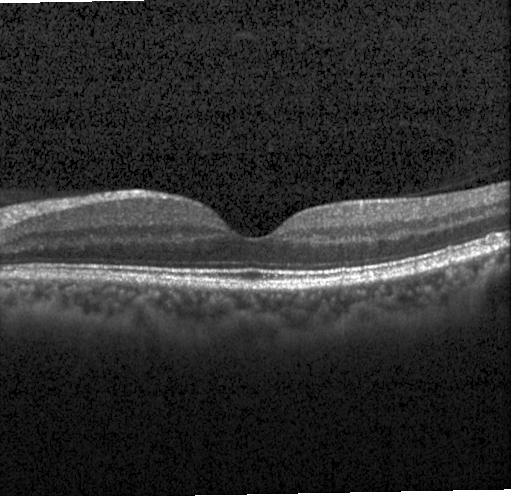
OCT scan showing neither choroidal neovascularization, diabetic macular edema, nor drusen.